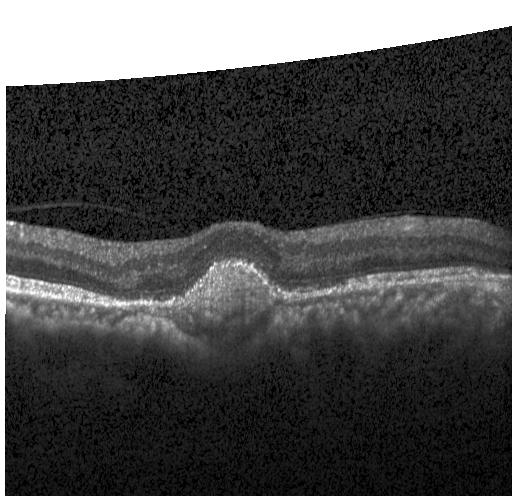
OCT B-scan · SD-OCT. Impression: choroidal neovascularization (CNV).